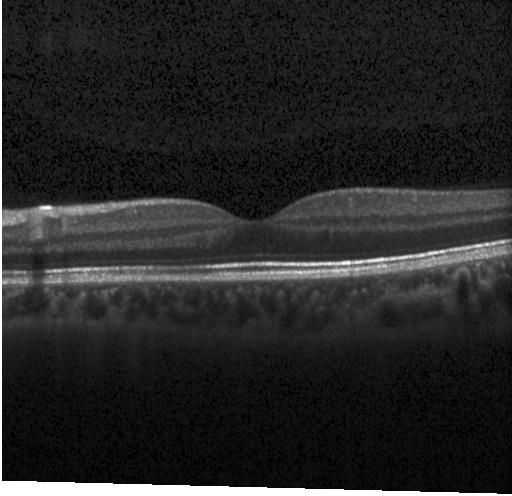
Optical coherence tomography scan. No choroidal neovascularization, no diabetic macular edema, and no drusen.